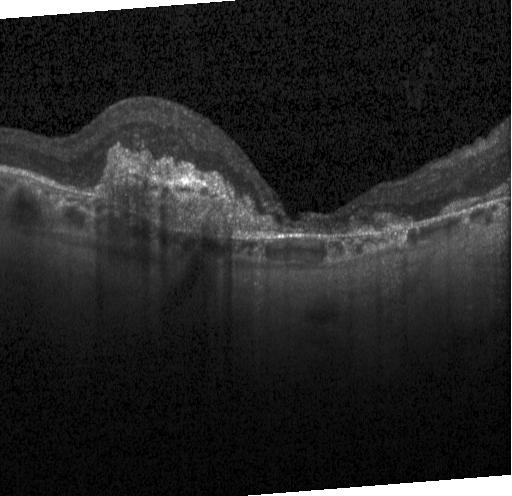 The scan shows choroidal neovascularization.